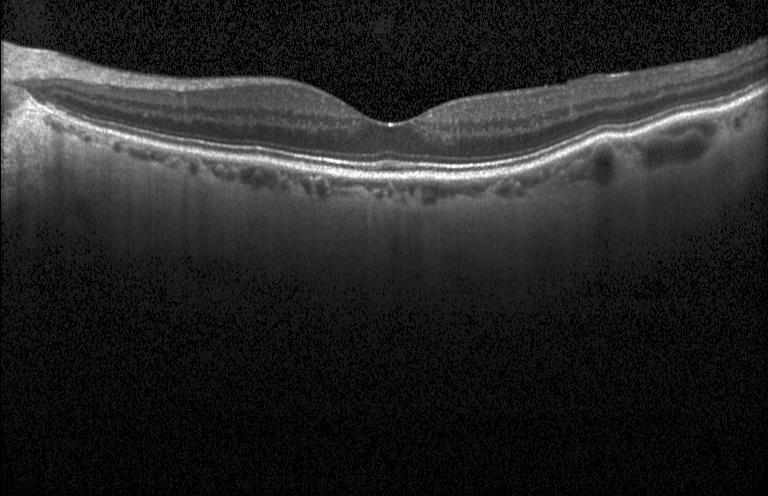

OCT B-scan. Heidelberg Spectralis. Horizontal scan through the fovea
Finding: no evidence of choroidal neovascularization, diabetic macular edema, or drusen.